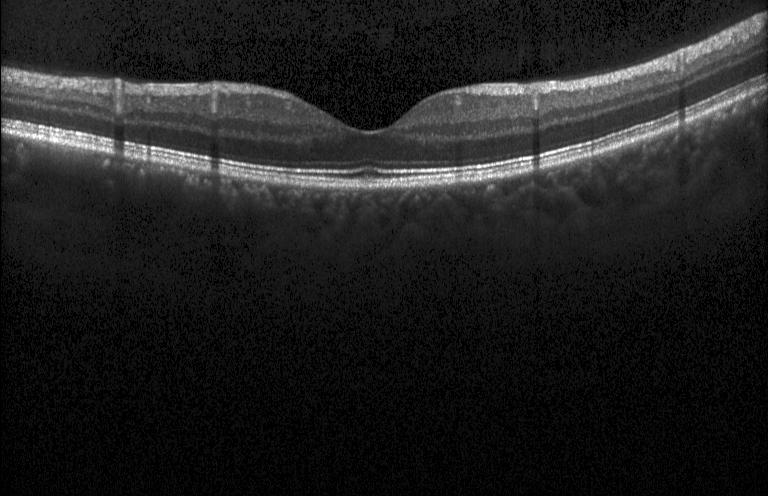 Impression: no choroidal neovascularization, no diabetic macular edema, and no drusen.